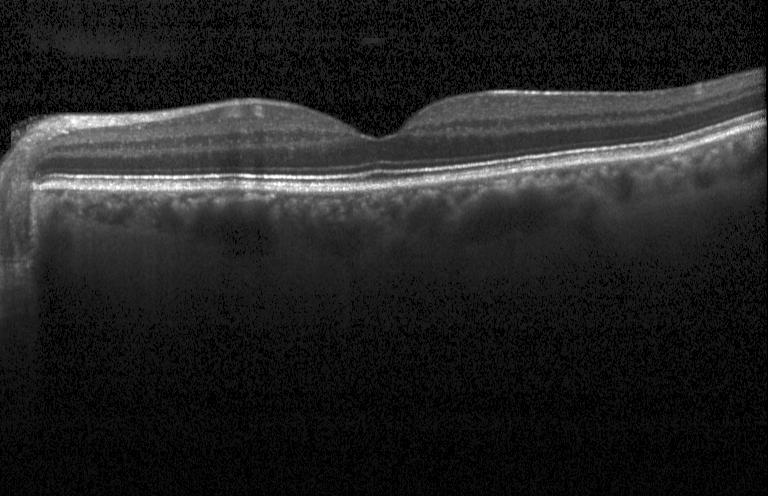

Spectral-domain OCT, retinal OCT cross-section, horizontal scan through the fovea, instrument: Heidelberg Spectralis — Assessment: no evidence of choroidal neovascularization, diabetic macular edema, or drusen.